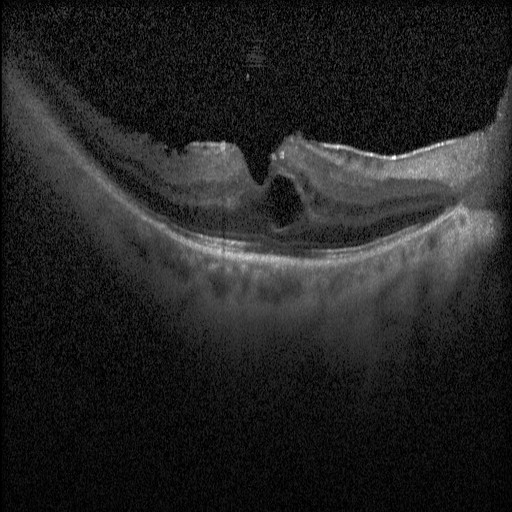 Spectral-domain OCT B-scan: diabetic macular edema.